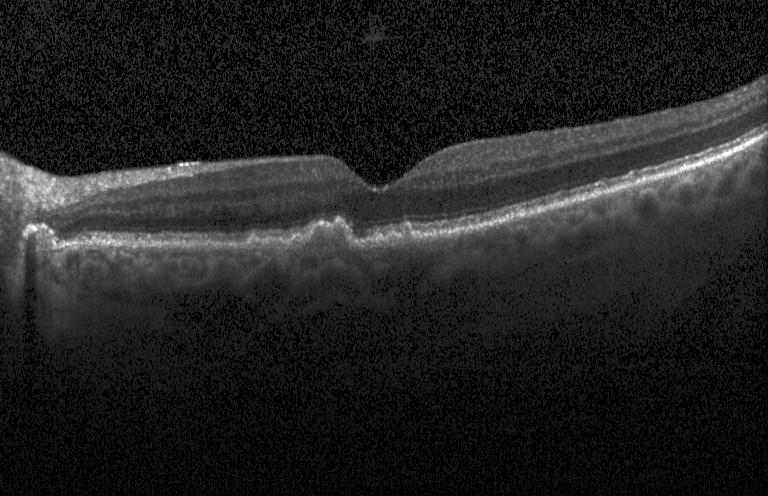

Finding: sub-RPE drusenoid deposits.